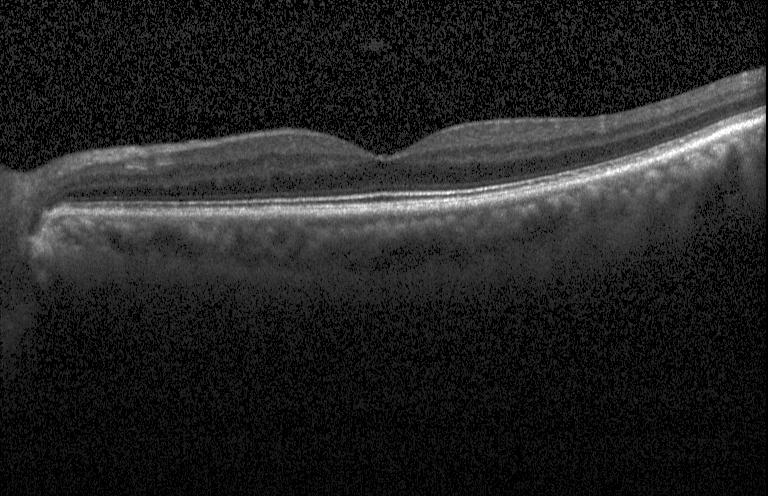

Optical coherence tomography B-scan.
Diagnosis: no CNV, no DME, and no drusen.